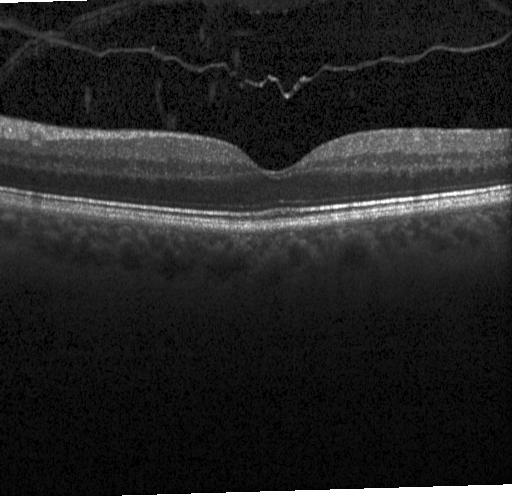
Macular OCT: no evidence of choroidal neovascularization, diabetic macular edema, or drusen.